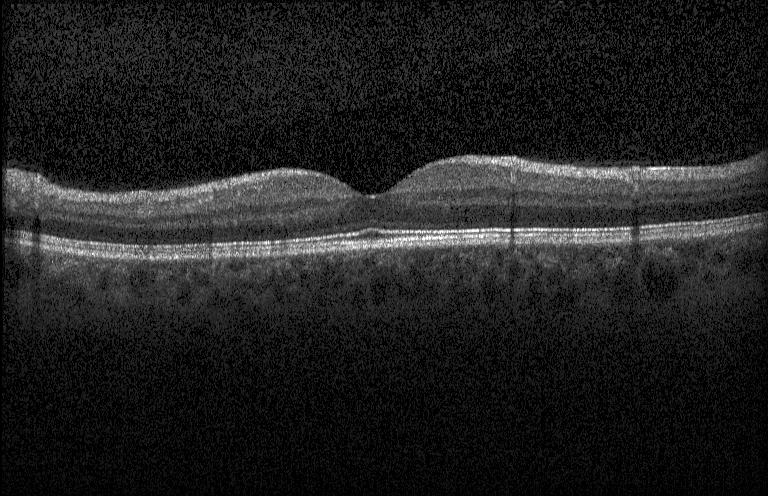

No choroidal neovascularization, diabetic macular edema, or drusen.